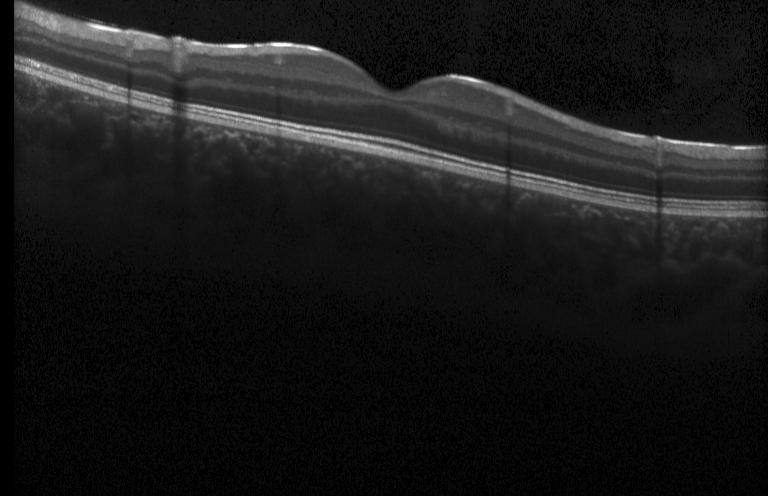 Macular OCT demonstrating neither choroidal neovascularization, diabetic macular edema, nor drusen.